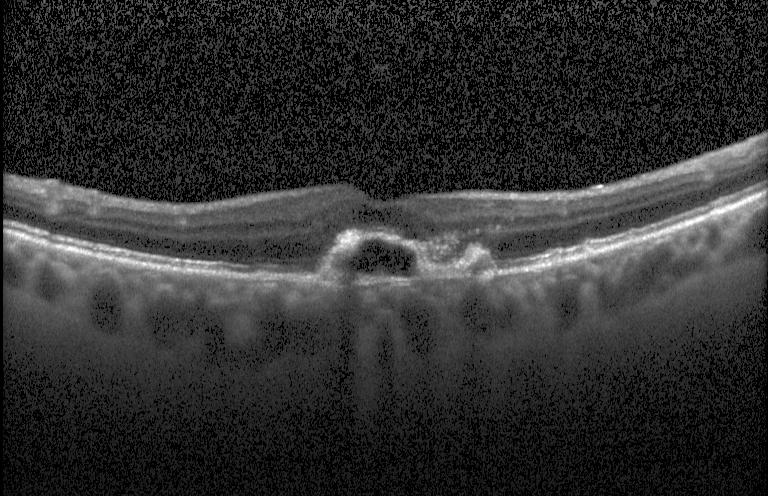

Optical coherence tomography scan · acquired on a Heidelberg Spectralis · spectral-domain OCT. The scan shows a choroidal neovascular membrane.